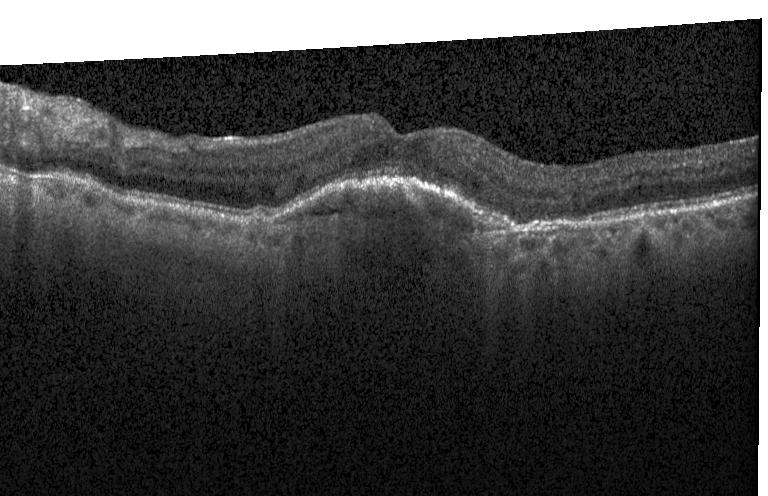
Assessment: a choroidal neovascular membrane.